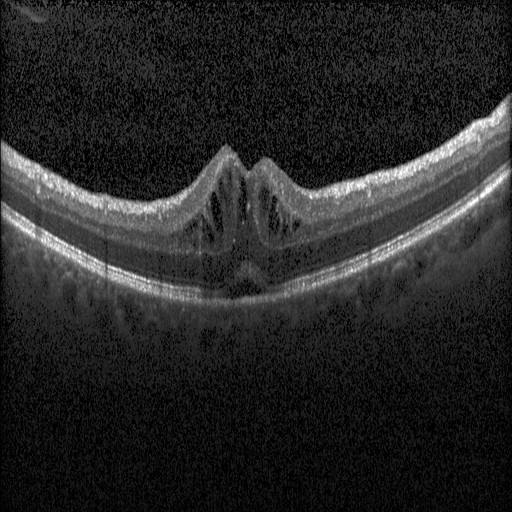
Diagnosis: DME.